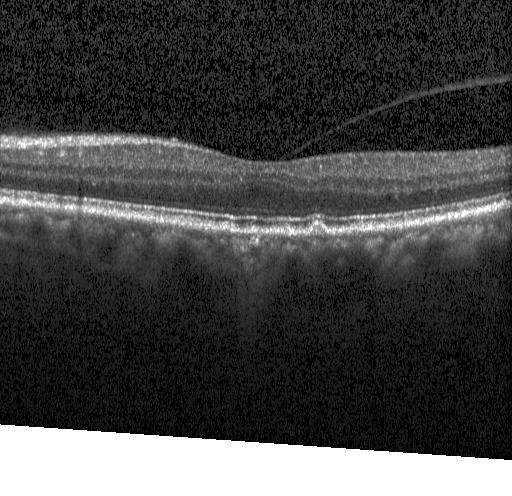

OCT scan showing drusen.